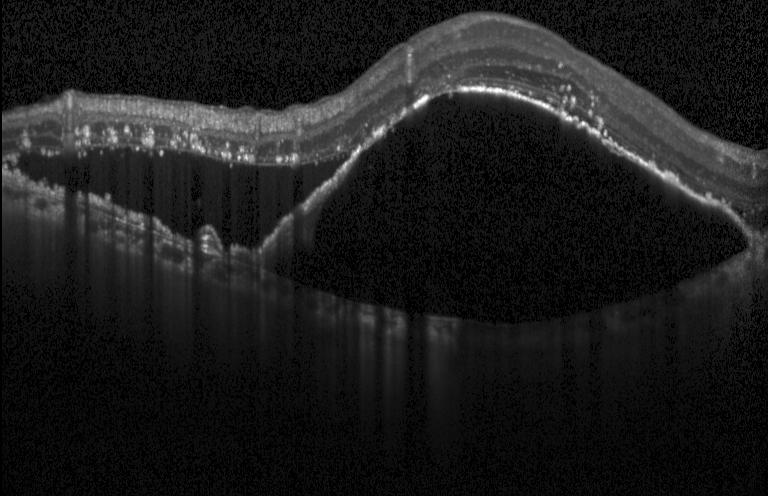
Optical coherence tomography B-scan, macular scan, Heidelberg Spectralis, spectral-domain OCT — Diagnosis: choroidal neovascularization (CNV).